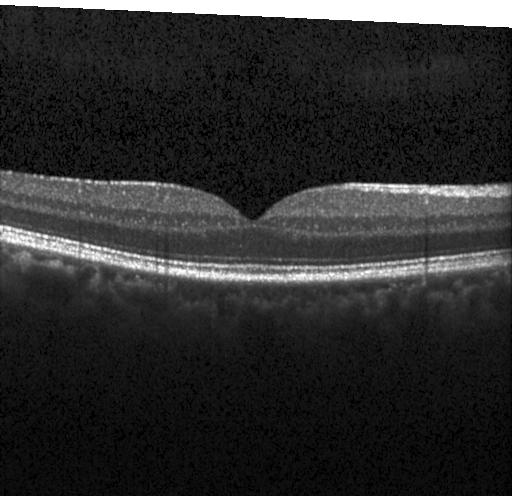
Acquired on a Heidelberg Spectralis; macular scan; optical coherence tomography scan
Diagnosis: no CNV, no DME, and no drusen.